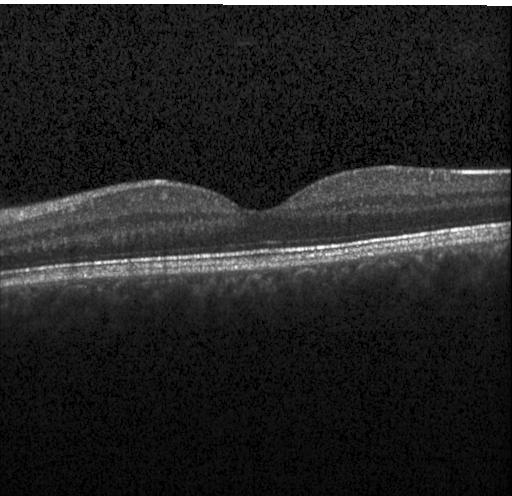

Macular OCT: no evidence of choroidal neovascularization, diabetic macular edema, or drusen.